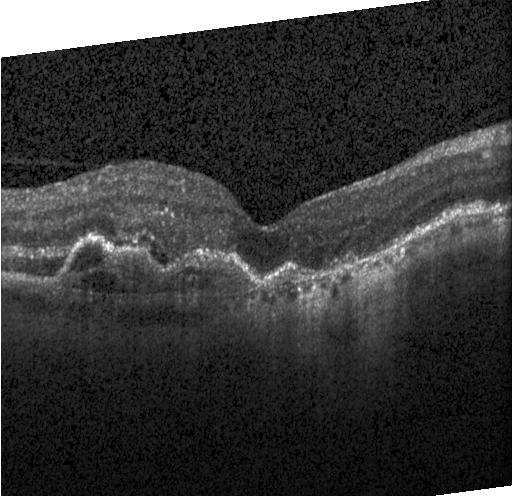 Optical coherence tomography B-scan. Impression: choroidal neovascularization (CNV).